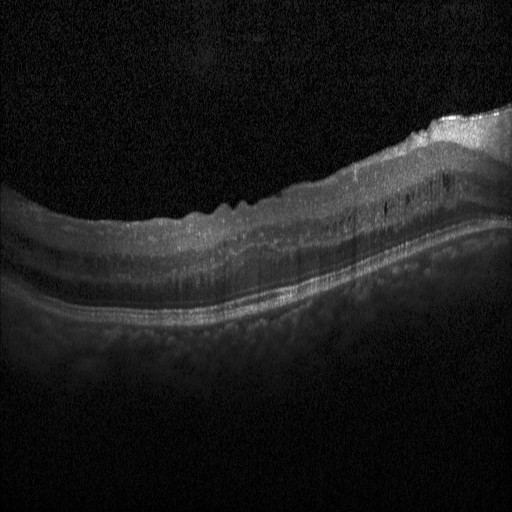 Impression: diabetic macular edema (DME).